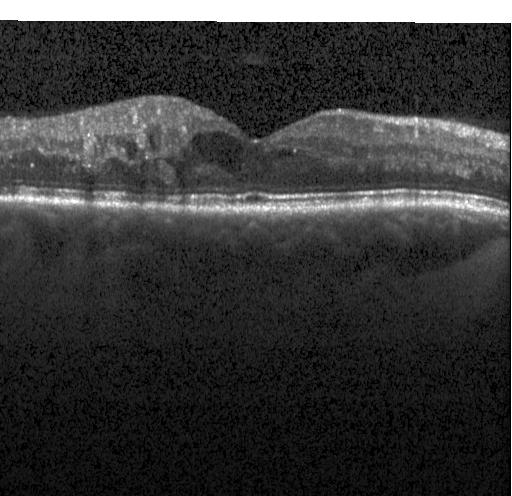
Dx: diabetic macular edema.